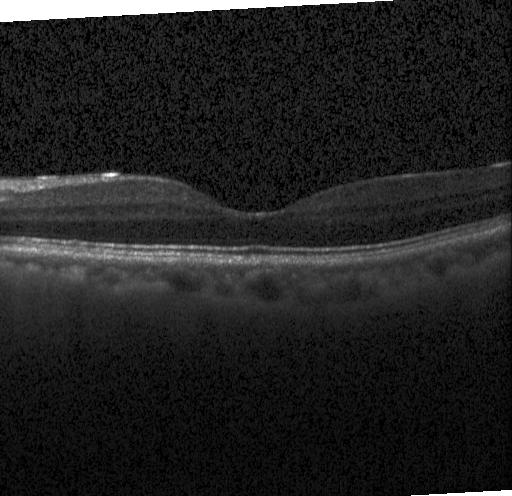

OCT line scan. Through the macula — Dx: no evidence of choroidal neovascularization, diabetic macular edema, or drusen.